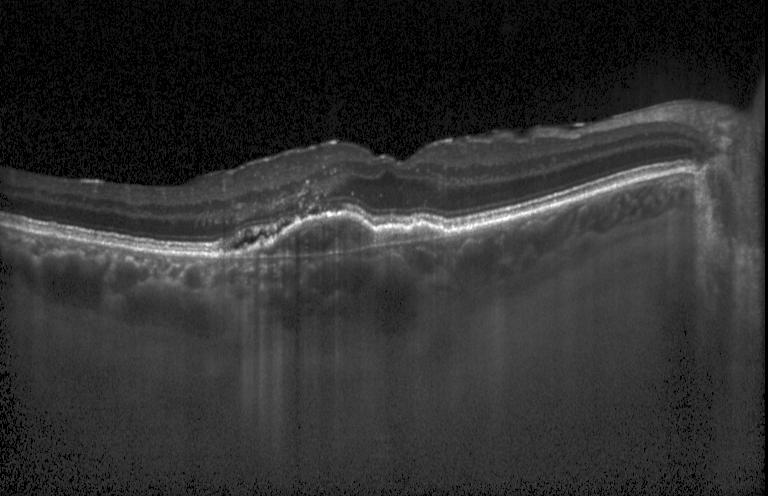

Spectral-domain OCT. Acquired on a Heidelberg Spectralis. Fovea-centered. OCT B-scan — Finding: choroidal neovascularization (CNV).